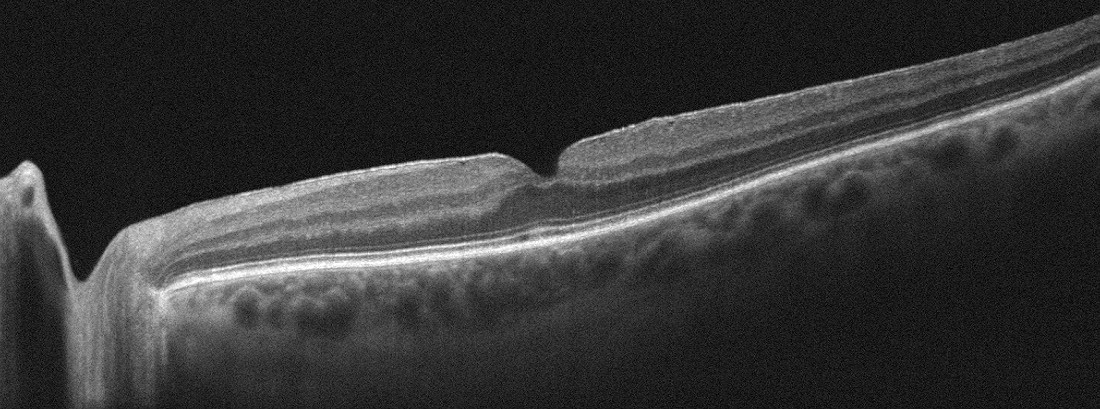 Impression: epiretinal membrane.